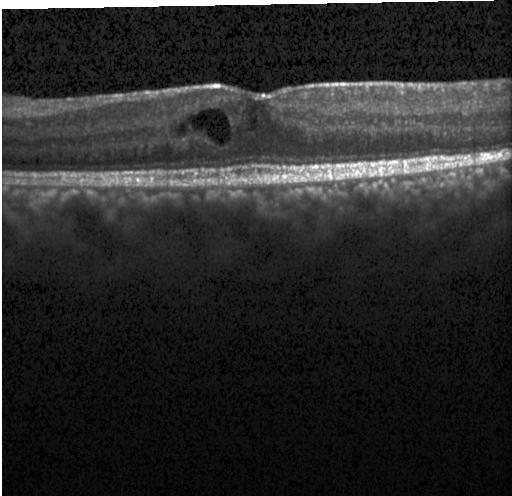 Macular OCT demonstrating DME.